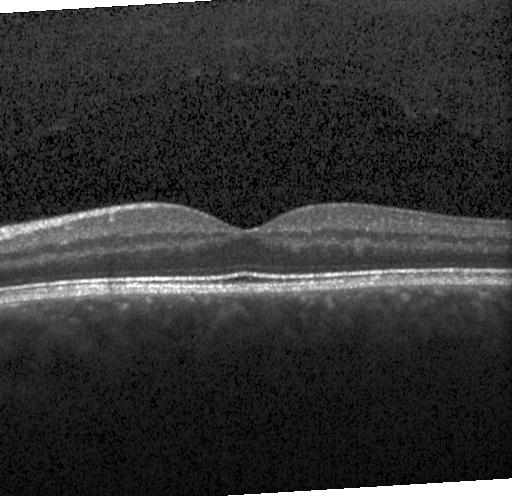
Horizontal scan through the fovea, optical coherence tomography scan
Dx: no evidence of choroidal neovascularization, diabetic macular edema, or drusen.